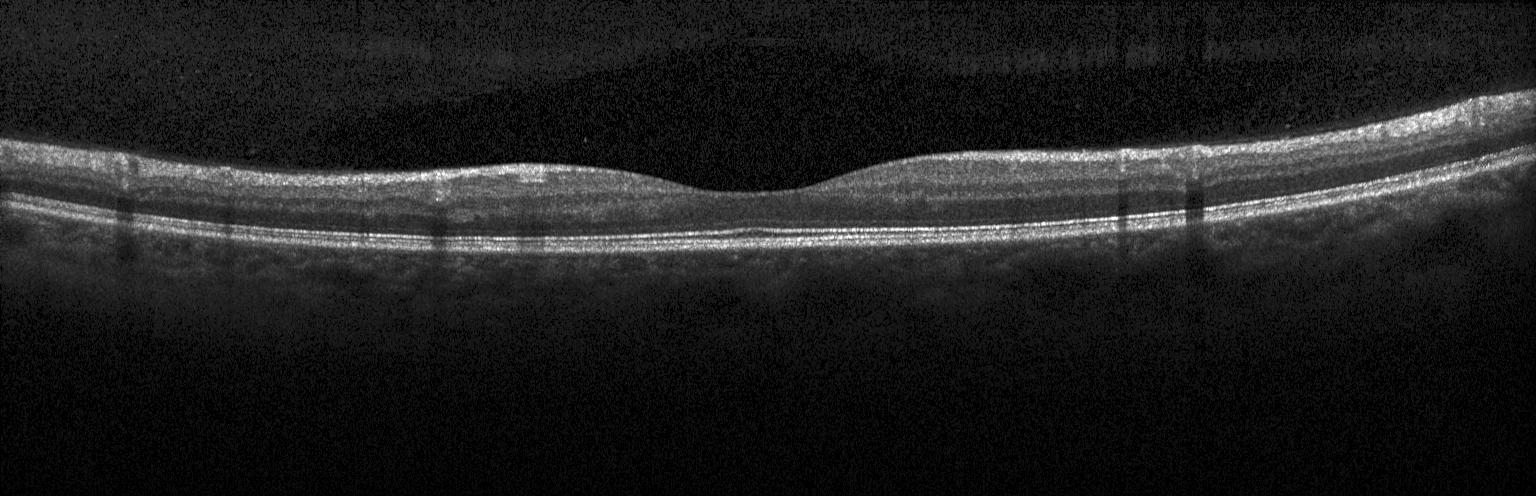

Heidelberg Spectralis OCT system. Retinal OCT cross-section. Macular scan
Diagnosis: no evidence of CNV, DME, or drusen.